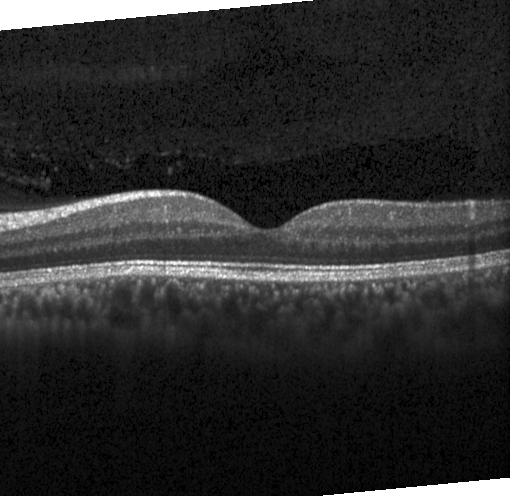

Instrument: Heidelberg Spectralis; centered on the fovea; retinal OCT cross-section. Diagnosis: no CNV, DME, or drusen.